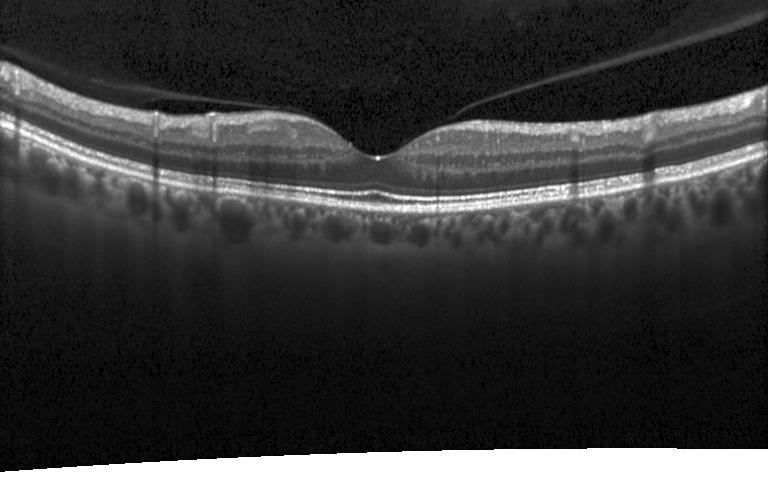
Diagnosis: no choroidal neovascularization, diabetic macular edema, or drusen.